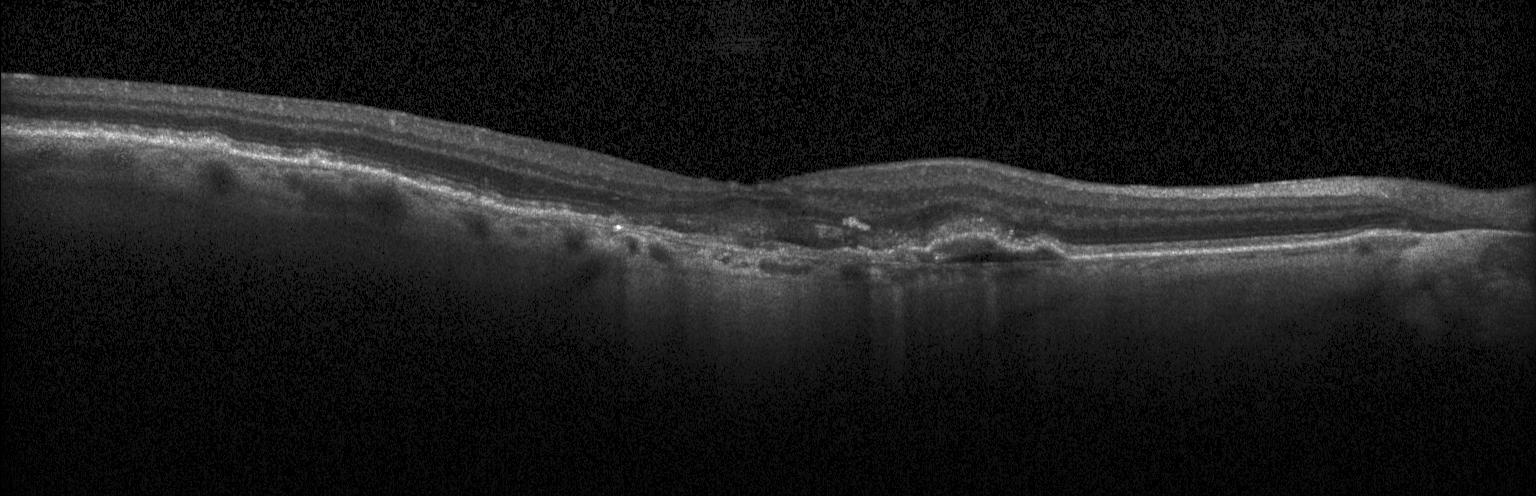
Retinal OCT cross-section showing choroidal neovascularization (CNV).